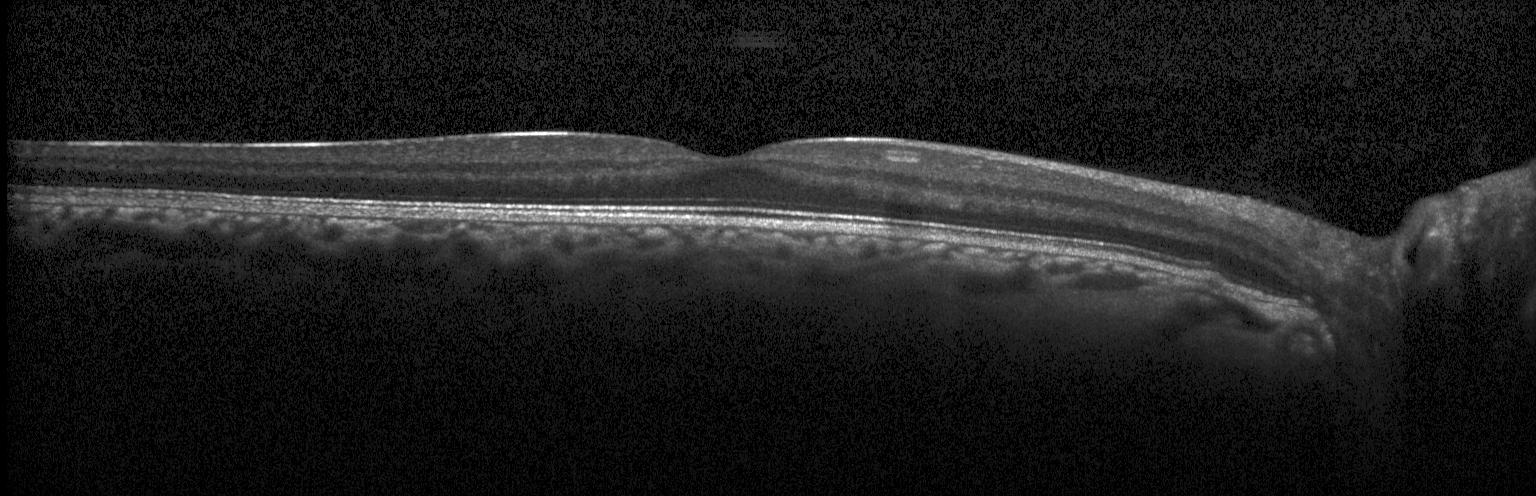

Acquired on a Heidelberg Spectralis, through the macula, optical coherence tomography B-scan, spectral-domain optical coherence tomography. Assessment: no choroidal neovascularization, diabetic macular edema, or drusen.